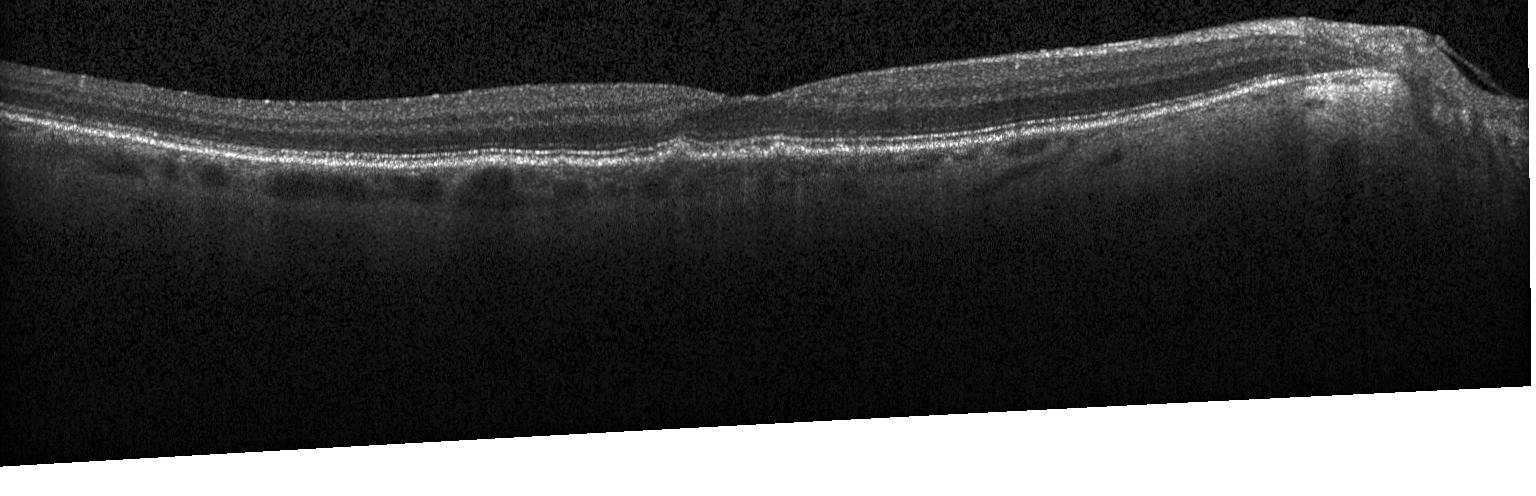 OCT line scan.
Assessment: drusen.